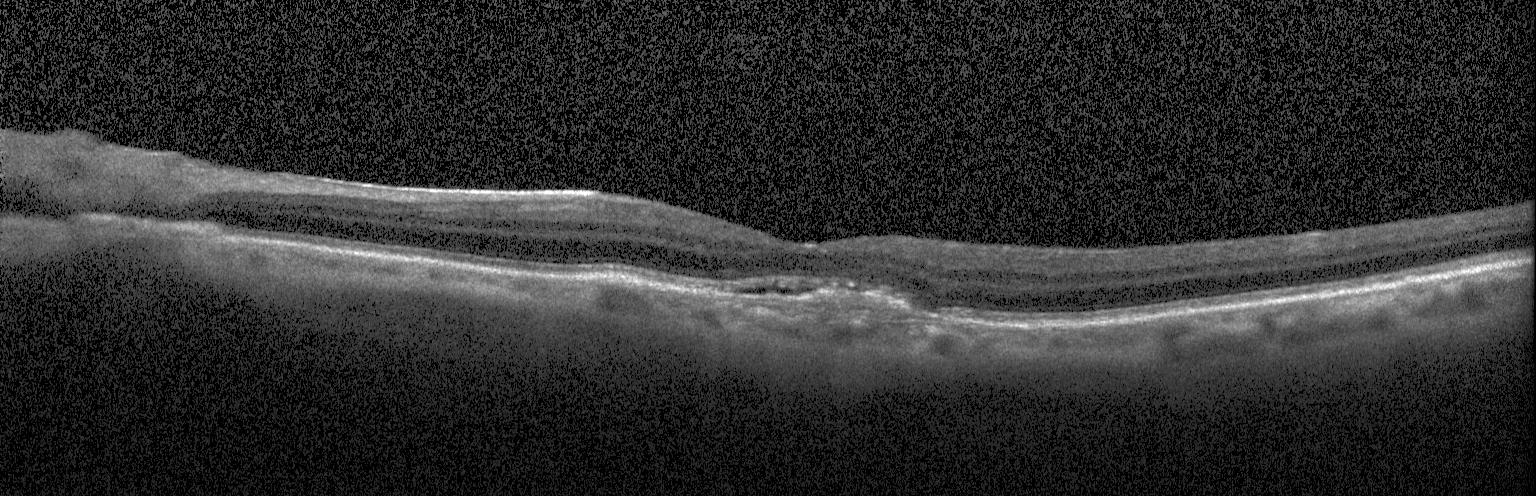
Acquired on a Heidelberg Spectralis. Retinal OCT cross-section. Spectral-domain optical coherence tomography. Diagnosis: choroidal neovascularization.